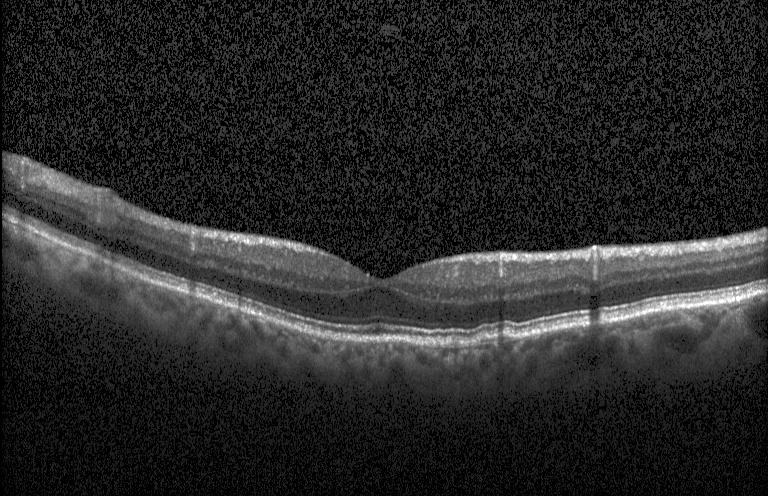
Retinal OCT cross-section · Heidelberg Spectralis · horizontal scan through the fovea.
Finding: sub-RPE drusenoid deposits.